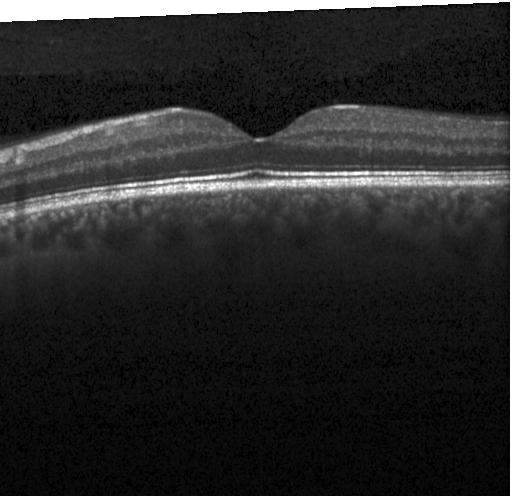 Diagnosis: neither choroidal neovascularization, diabetic macular edema, nor drusen.